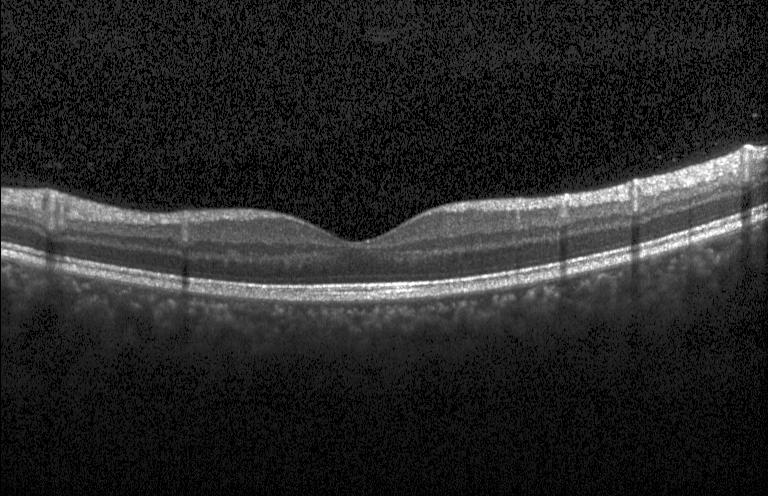
Heidelberg Spectralis. Optical coherence tomography B-scan. Centered on the fovea. SD-OCT.
Macular OCT: neither CNV, DME, nor drusen.